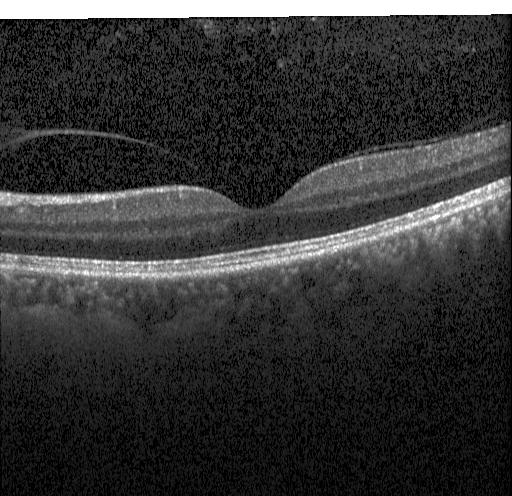

Impression: no evidence of CNV, DME, or drusen.